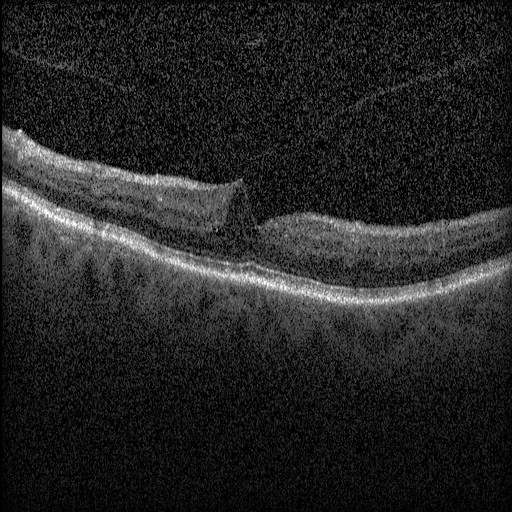 Retinal OCT cross-section showing diabetic macular edema (DME).